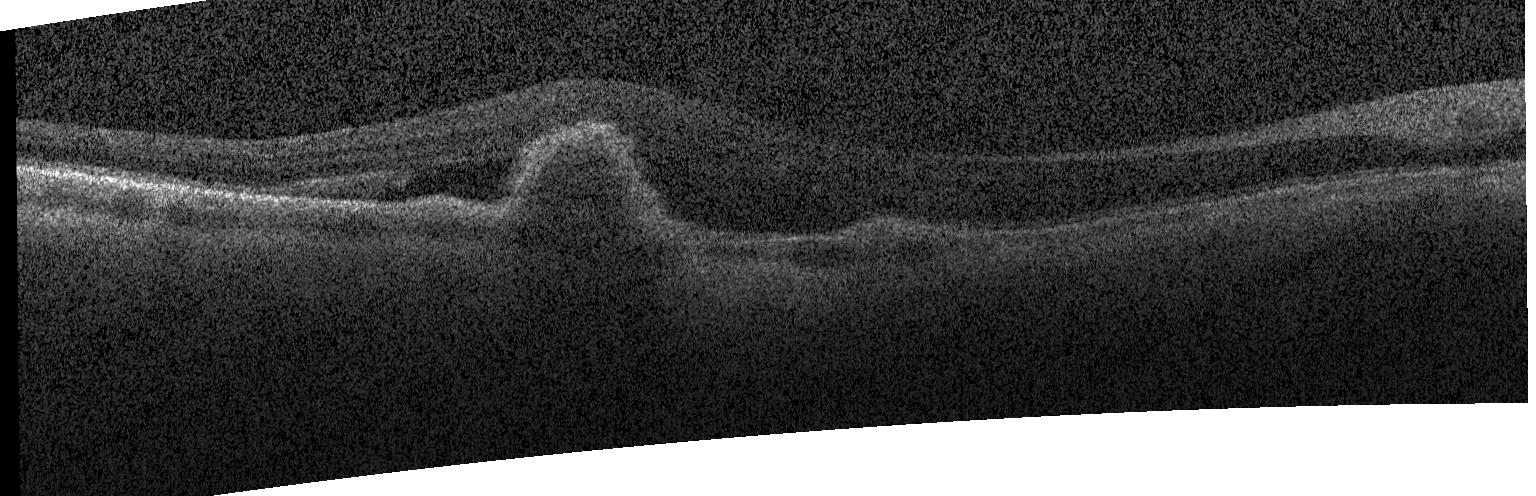 SD-OCT. Retinal OCT cross-section. Through the macula. Instrument: Heidelberg Spectralis
Assessment: choroidal neovascularization.